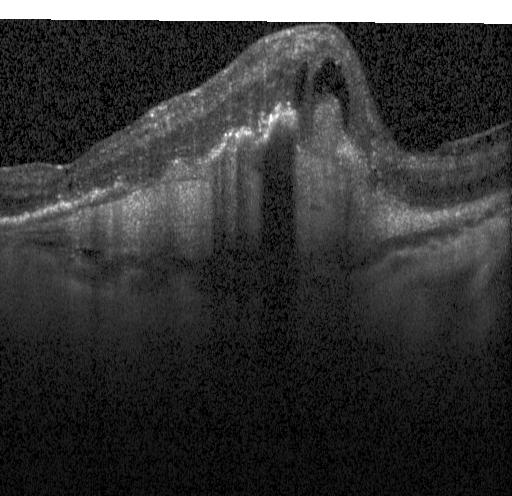 Dx: a choroidal neovascular membrane.